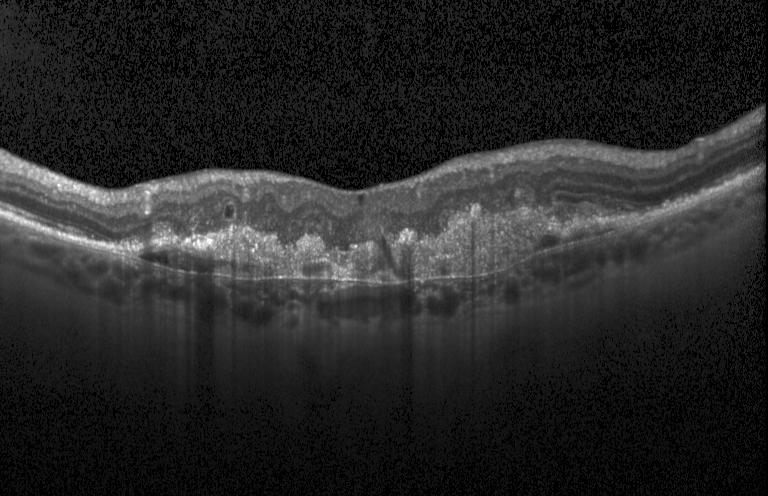 Spectral-domain optical coherence tomography. OCT line scan
The scan shows CNV.